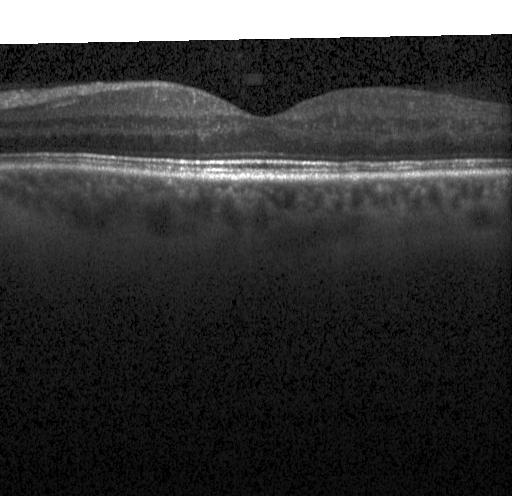

OCT B-scan
Assessment: no choroidal neovascularization, no diabetic macular edema, and no drusen.